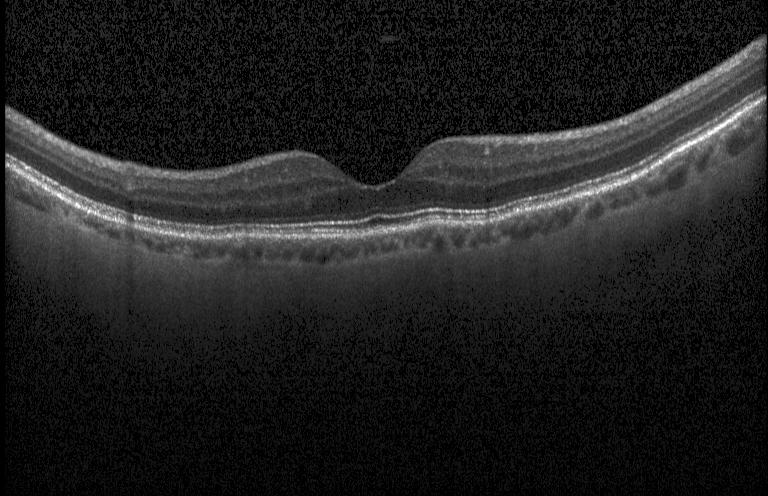
Retinal OCT cross-section · SD-OCT.
Dx: no choroidal neovascularization, no diabetic macular edema, and no drusen.